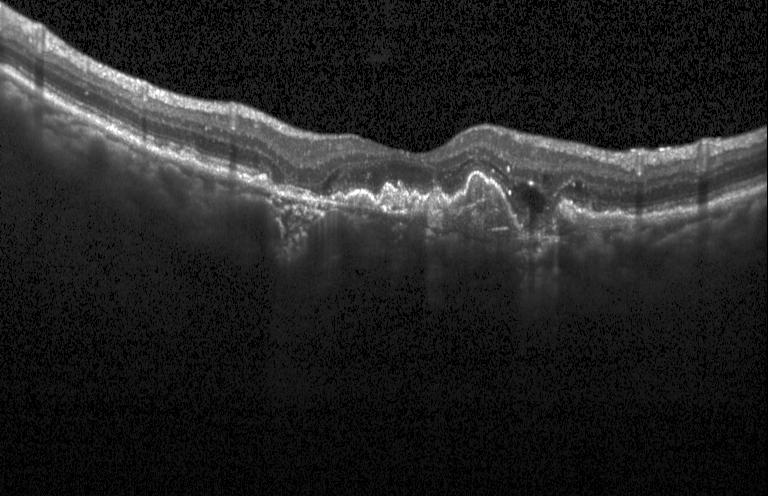

Retinal OCT B-scan, Heidelberg Spectralis
Finding: CNV.